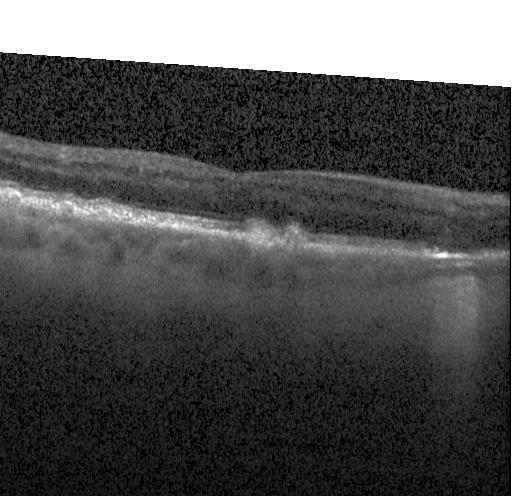 Spectral-domain OCT B-scan: drusen.